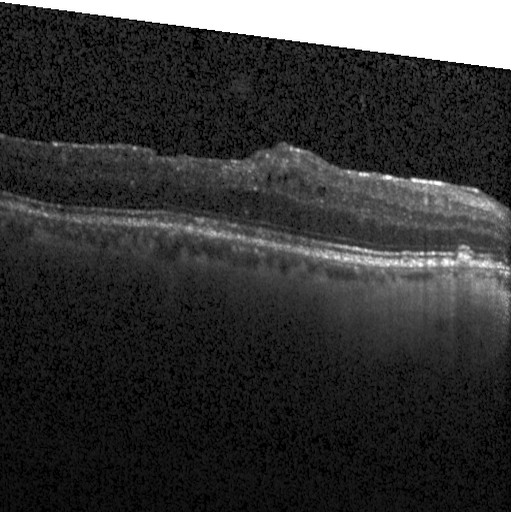
Macular scan · OCT B-scan · spectral-domain OCT
Impression: diabetic macular edema.